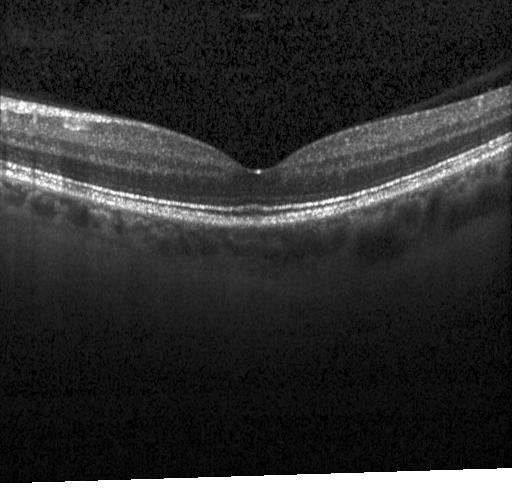 Optical coherence tomography scan
Diagnosis: no evidence of choroidal neovascularization, diabetic macular edema, or drusen.